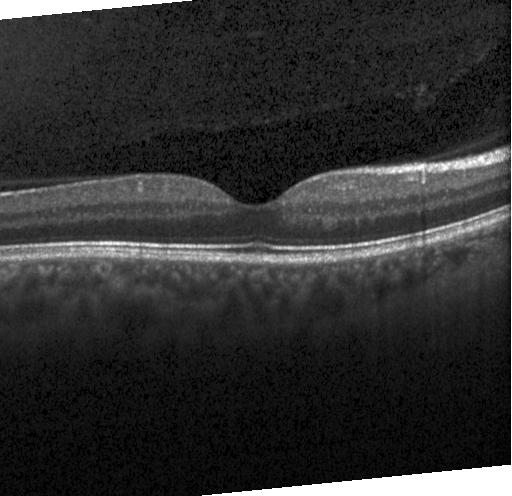

Retinal OCT cross-section. Heidelberg Spectralis — Assessment: neither choroidal neovascularization, diabetic macular edema, nor drusen.